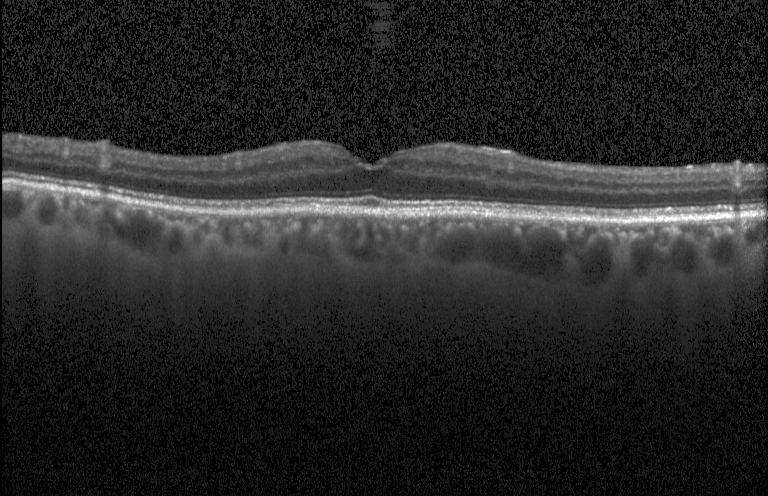

Through the macula. Spectral-domain optical coherence tomography. Instrument: Heidelberg Spectralis. Retinal OCT cross-section — Assessment: neither choroidal neovascularization, diabetic macular edema, nor drusen.